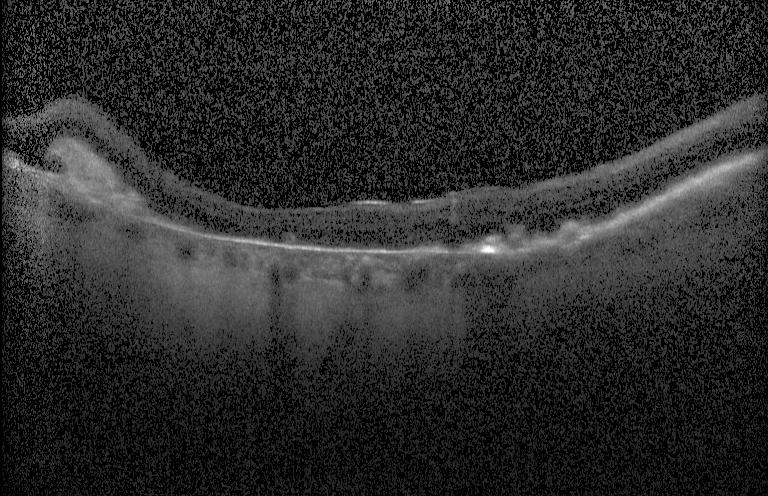 Through the macula. Optical coherence tomography B-scan — Macular OCT: CNV.